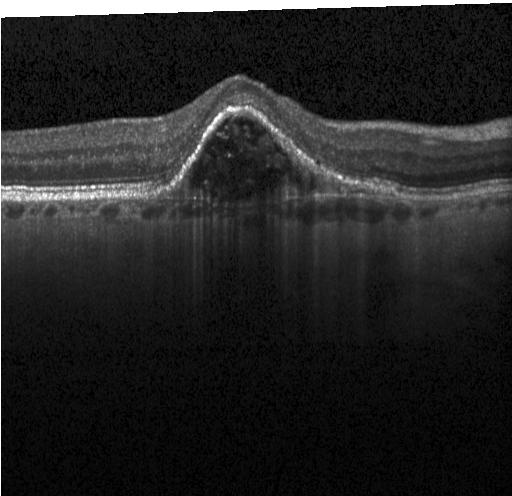

This B-scan demonstrates CNV.